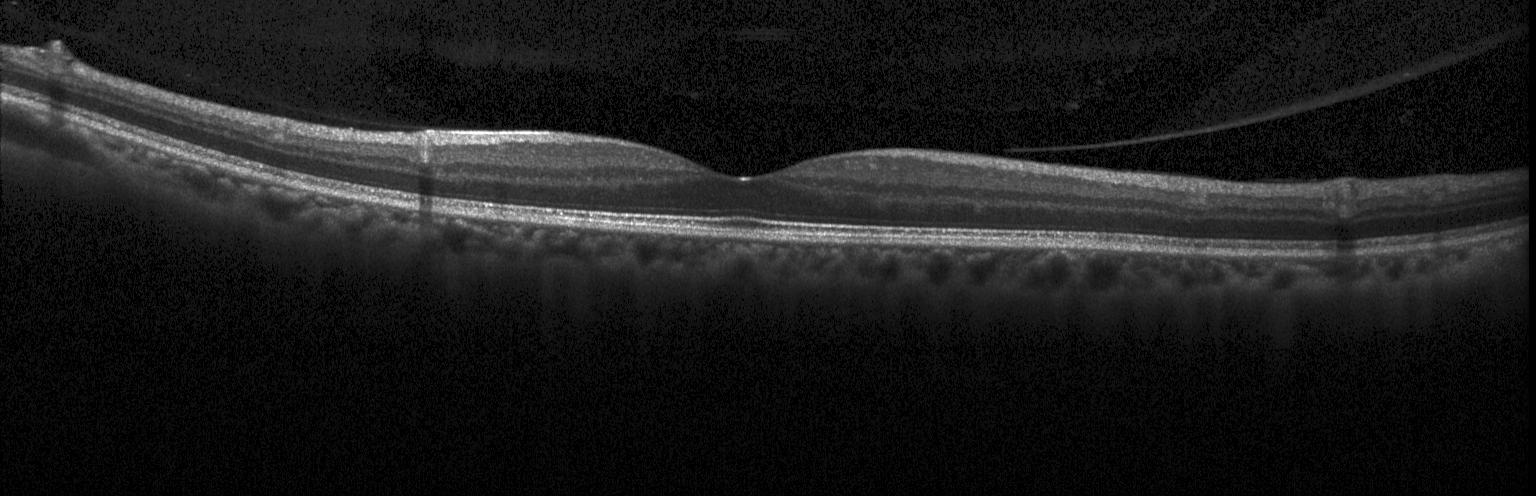 Retinal OCT B-scan. Centered on the fovea. Spectral-domain optical coherence tomography. Impression: no CNV, DME, or drusen.